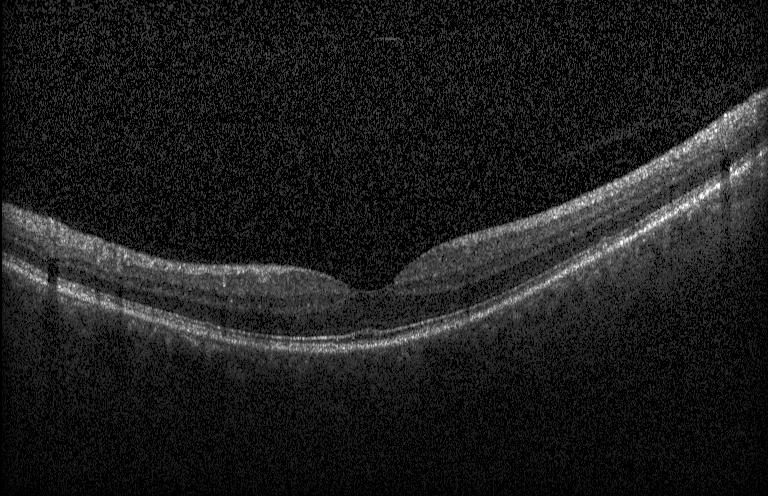

Optical coherence tomography B-scan. Diagnosis: no choroidal neovascularization, diabetic macular edema, or drusen.